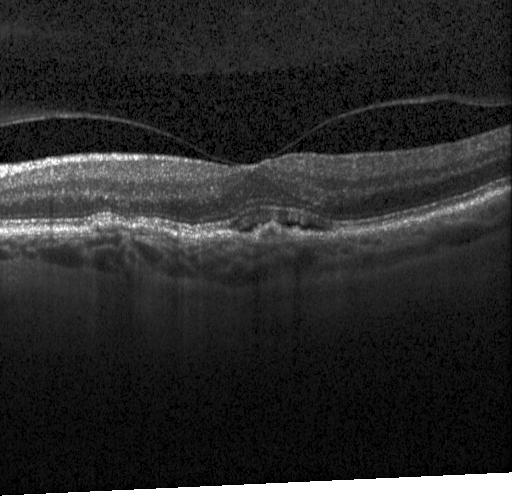

Macular OCT: CNV.